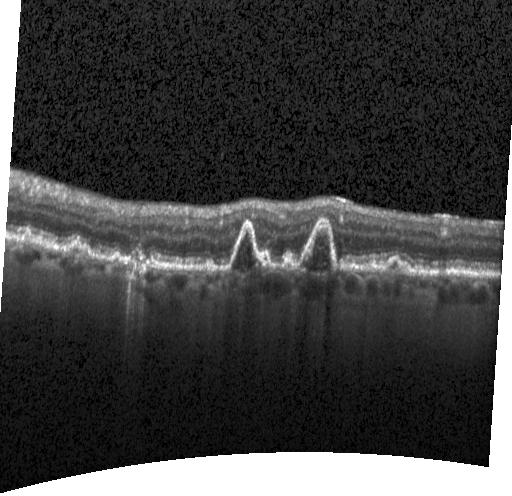 OCT line scan · fovea-centered — Diagnosis: CNV.